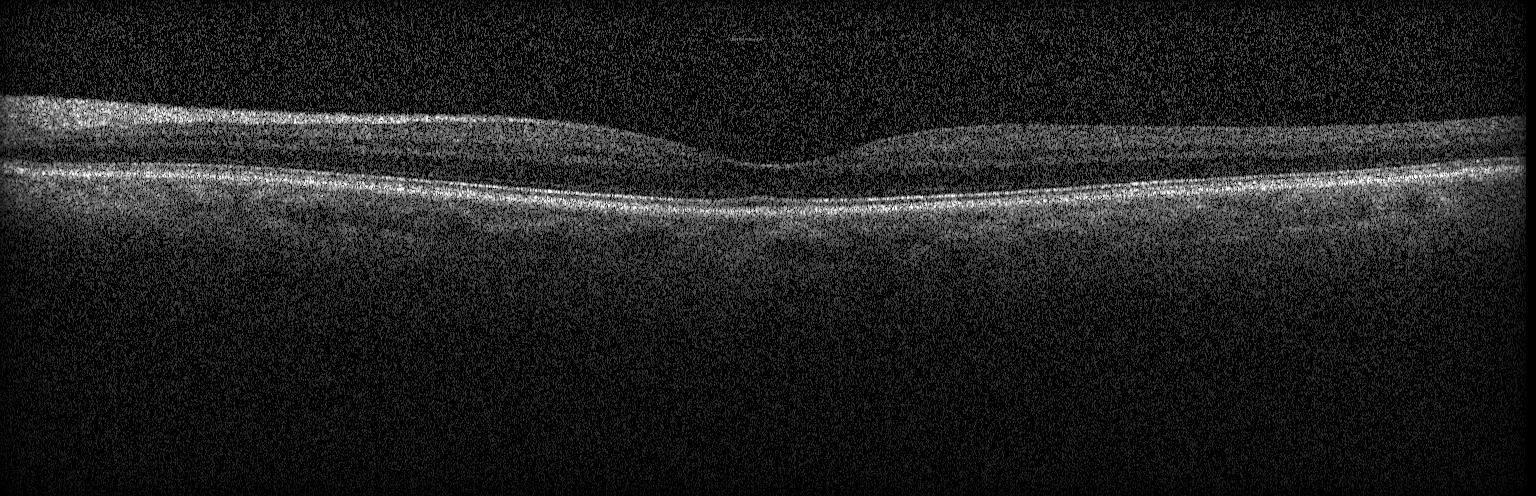 Retinal OCT B-scan · horizontal scan through the fovea
Impression: no evidence of choroidal neovascularization, diabetic macular edema, or drusen.